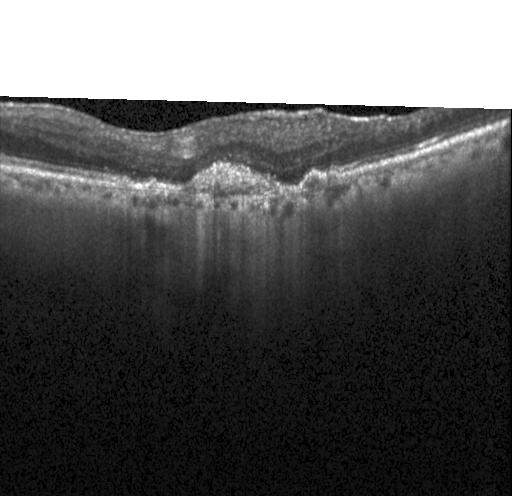 Choroidal neovascularization (CNV).